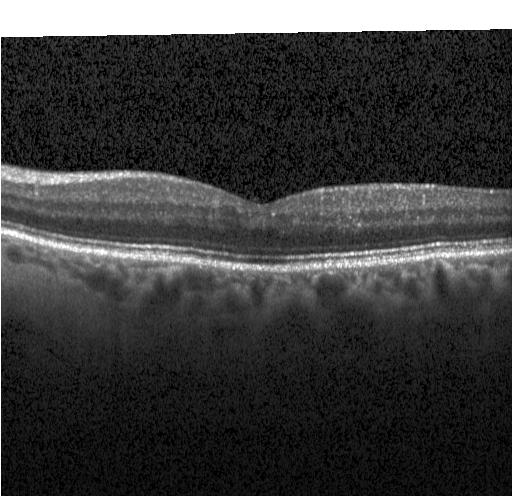
OCT B-scan. This B-scan demonstrates no CNV, DME, or drusen.